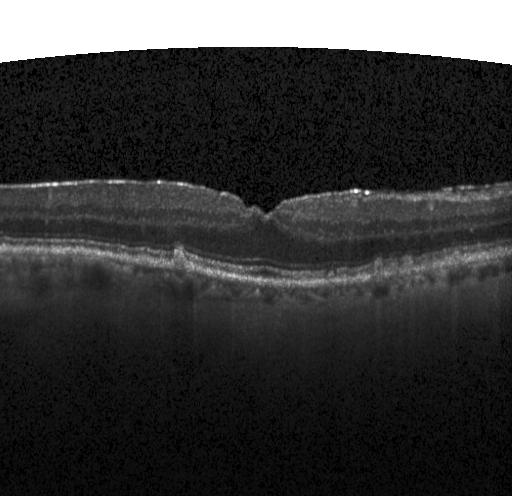 Spectral-domain optical coherence tomography · Heidelberg Spectralis · retinal OCT cross-section · centered on the fovea.
The scan shows sub-RPE drusenoid deposits.